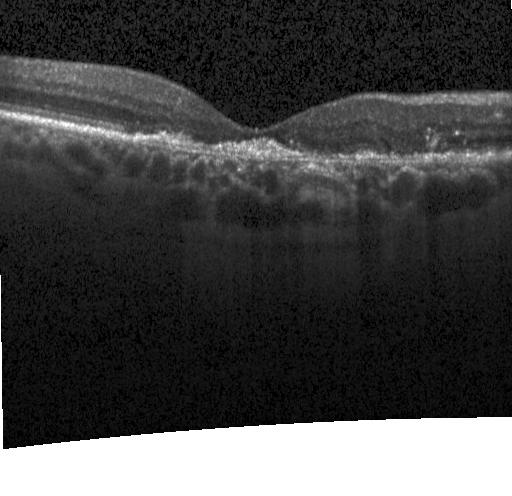

OCT B-scan. SD-OCT. Through the macula
Finding: choroidal neovascularization (CNV).